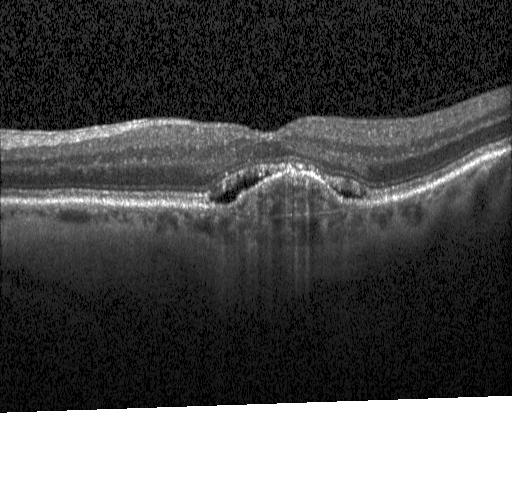

Instrument: Heidelberg Spectralis, retinal OCT B-scan, through the macula, SD-OCT. Dx: a choroidal neovascular membrane.